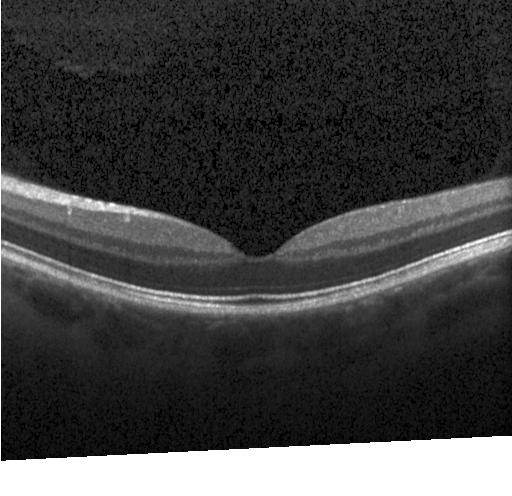 Macular OCT: neither choroidal neovascularization, diabetic macular edema, nor drusen.